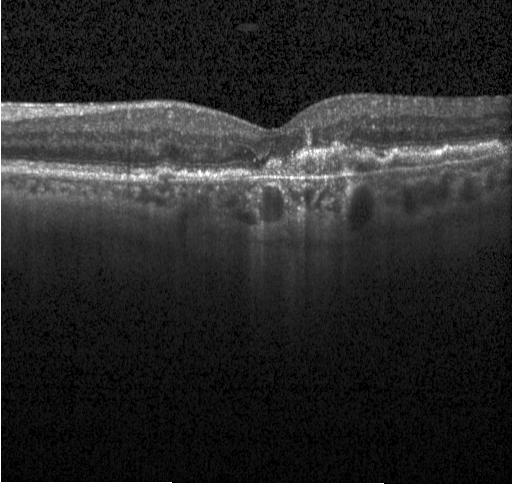 Retinal OCT cross-section — Impression: a choroidal neovascular membrane.